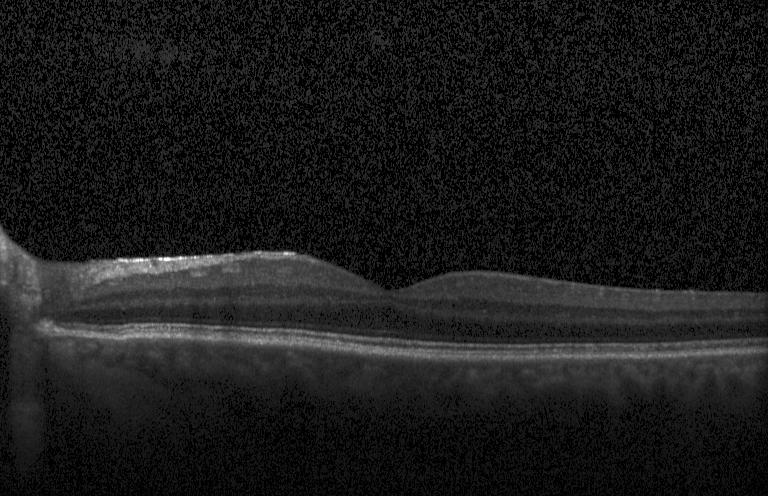
Instrument: Heidelberg Spectralis. Centered on the fovea. Optical coherence tomography scan. Spectral-domain OCT.
The scan shows no choroidal neovascularization, diabetic macular edema, or drusen.